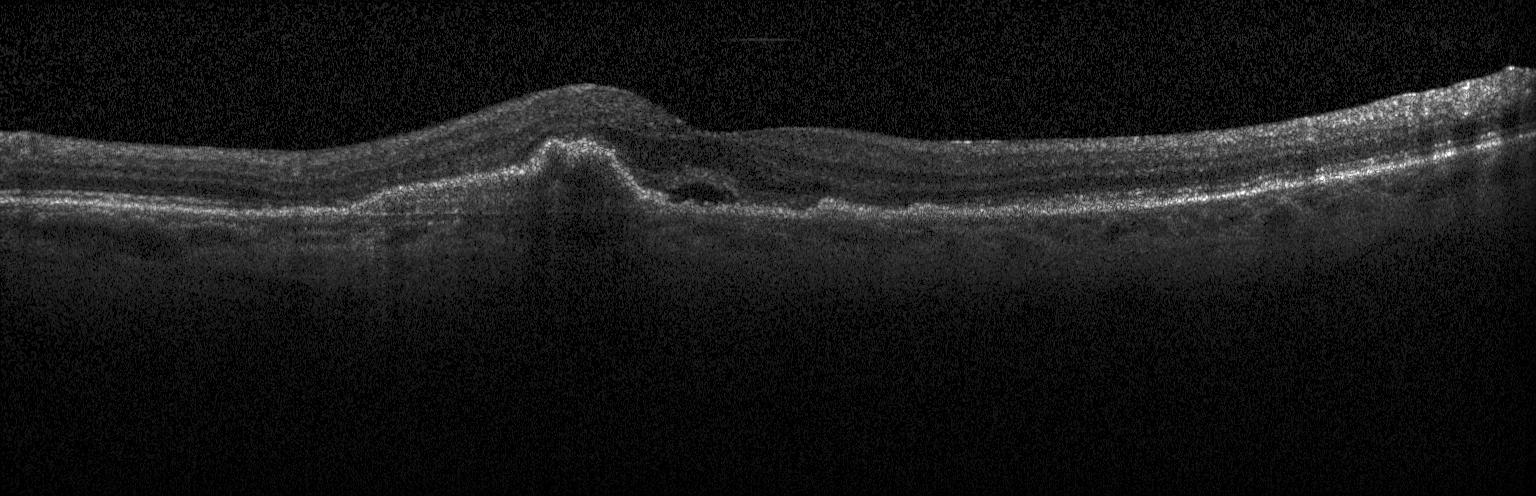
Retinal OCT cross-section showing a choroidal neovascular membrane.